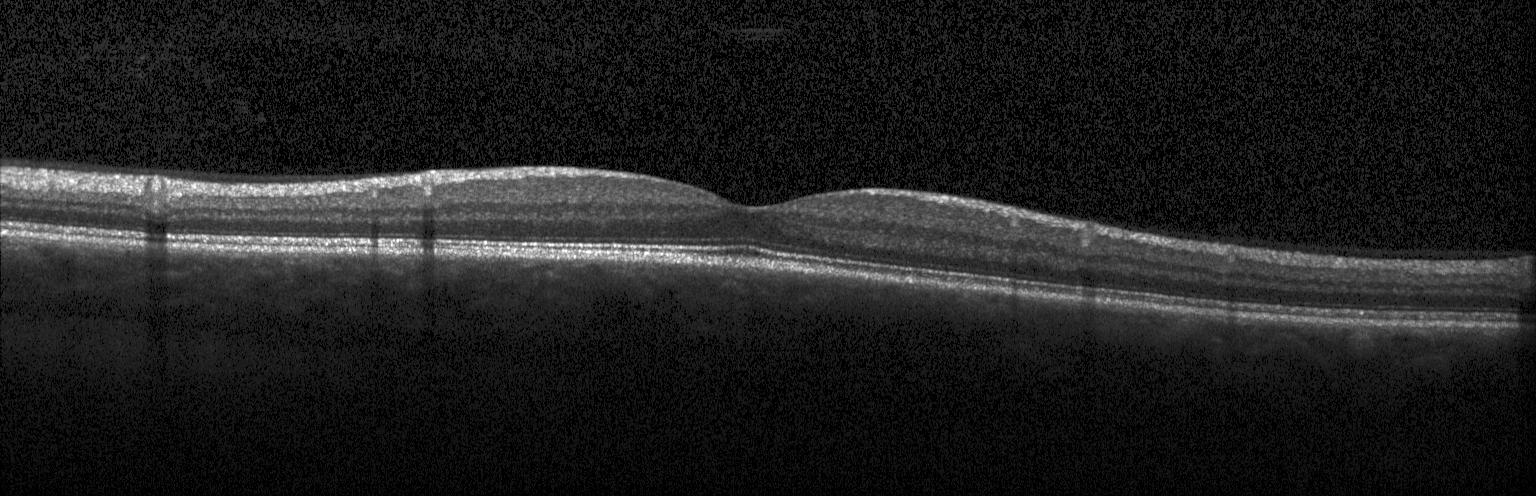

Diagnosis: no evidence of CNV, DME, or drusen.